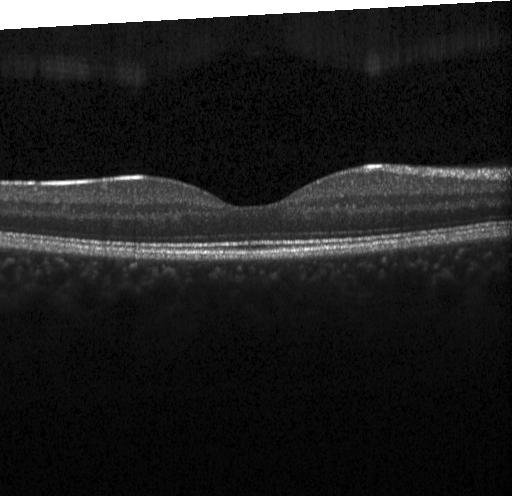

Dx: no evidence of choroidal neovascularization, diabetic macular edema, or drusen.